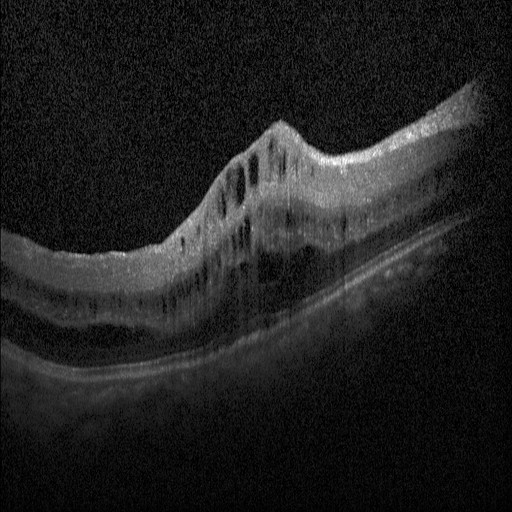

Impression: diabetic macular edema (DME).